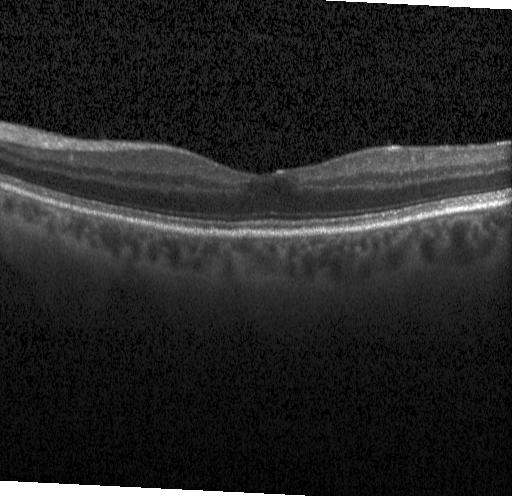
Optical coherence tomography B-scan · instrument: Heidelberg Spectralis · through the macula · spectral-domain OCT — Dx: no CNV, no DME, and no drusen.